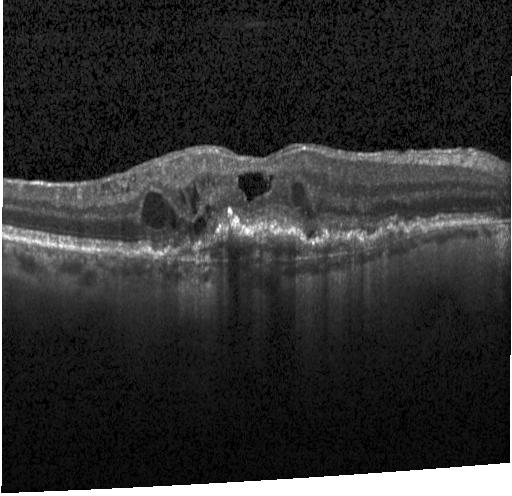
Optical coherence tomography B-scan, SD-OCT — Diagnosis: a choroidal neovascular membrane.